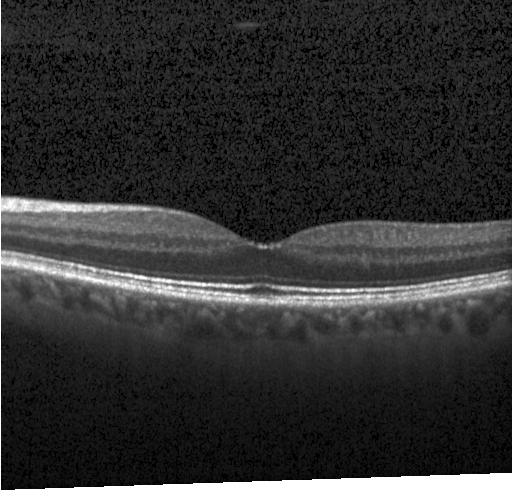 Retinal OCT cross-section showing no choroidal neovascularization, no diabetic macular edema, and no drusen.